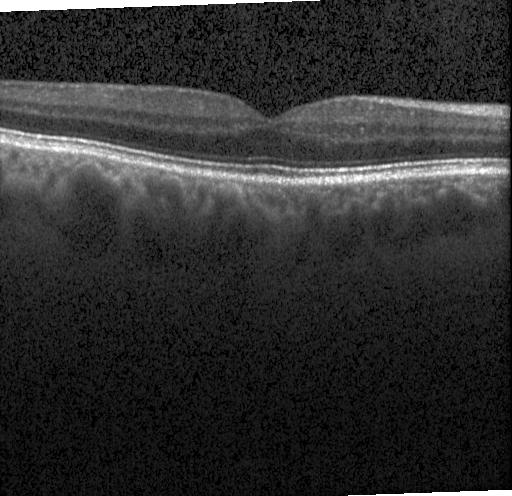 Heidelberg Spectralis OCT system; OCT B-scan; centered on the fovea. Dx: no choroidal neovascularization, diabetic macular edema, or drusen.